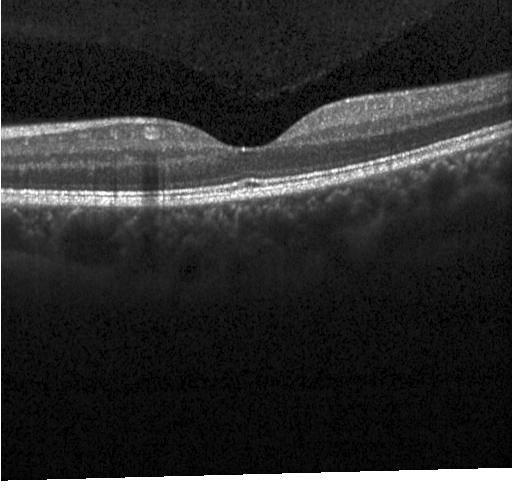
OCT B-scan showing no CNV, DME, or drusen.